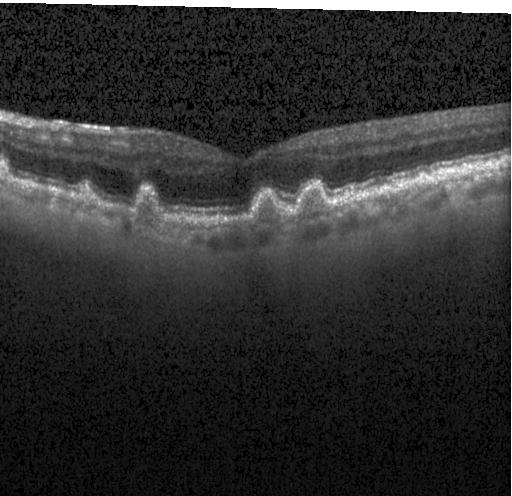 Finding: drusen.